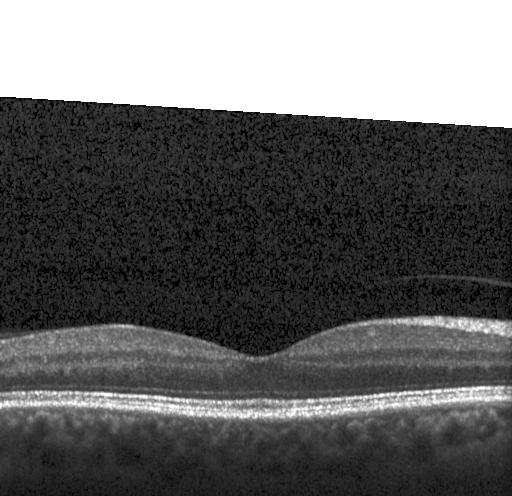

Retinal OCT cross-section · Heidelberg Spectralis · spectral-domain optical coherence tomography
Finding: no choroidal neovascularization, no diabetic macular edema, and no drusen.